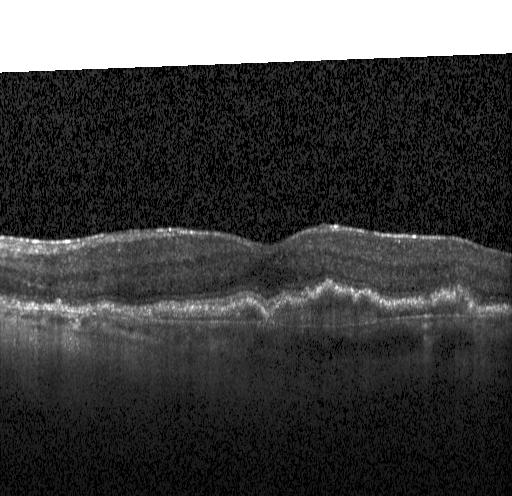

Spectral-domain optical coherence tomography · OCT line scan · macular scan · Heidelberg Spectralis
Dx: CNV.